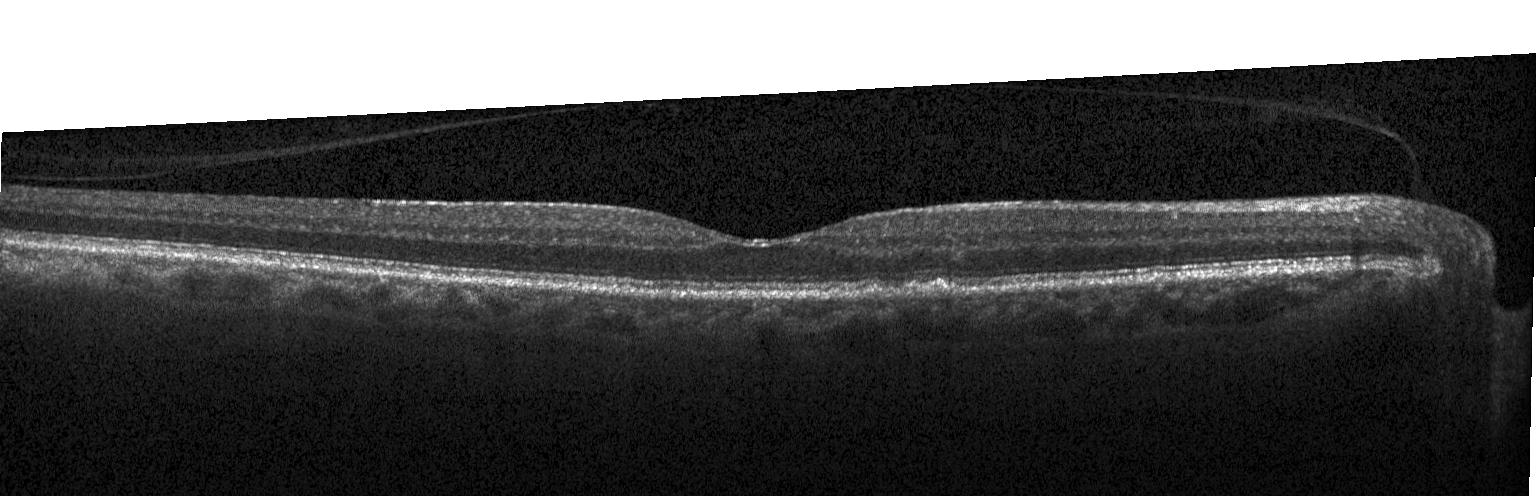
OCT B-scan. Sub-RPE drusenoid deposits.